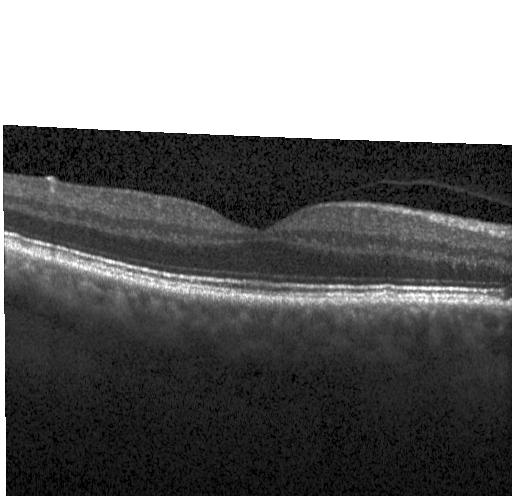
OCT finding: no CNV, DME, or drusen.